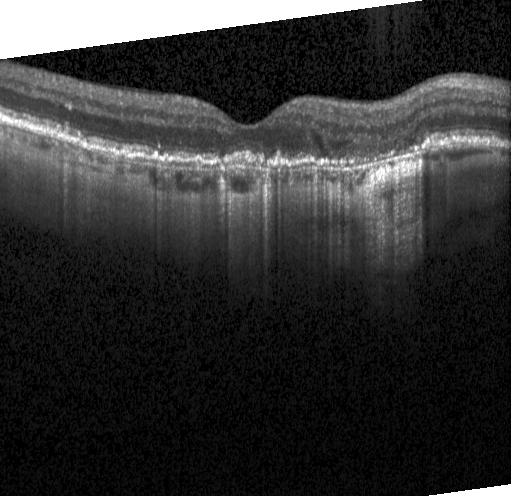
Macular OCT: choroidal neovascularization (CNV).